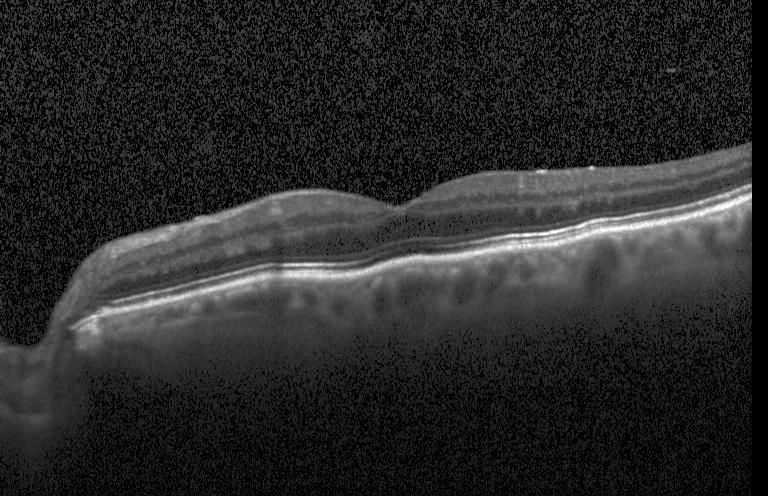
Impression: no evidence of choroidal neovascularization, diabetic macular edema, or drusen.